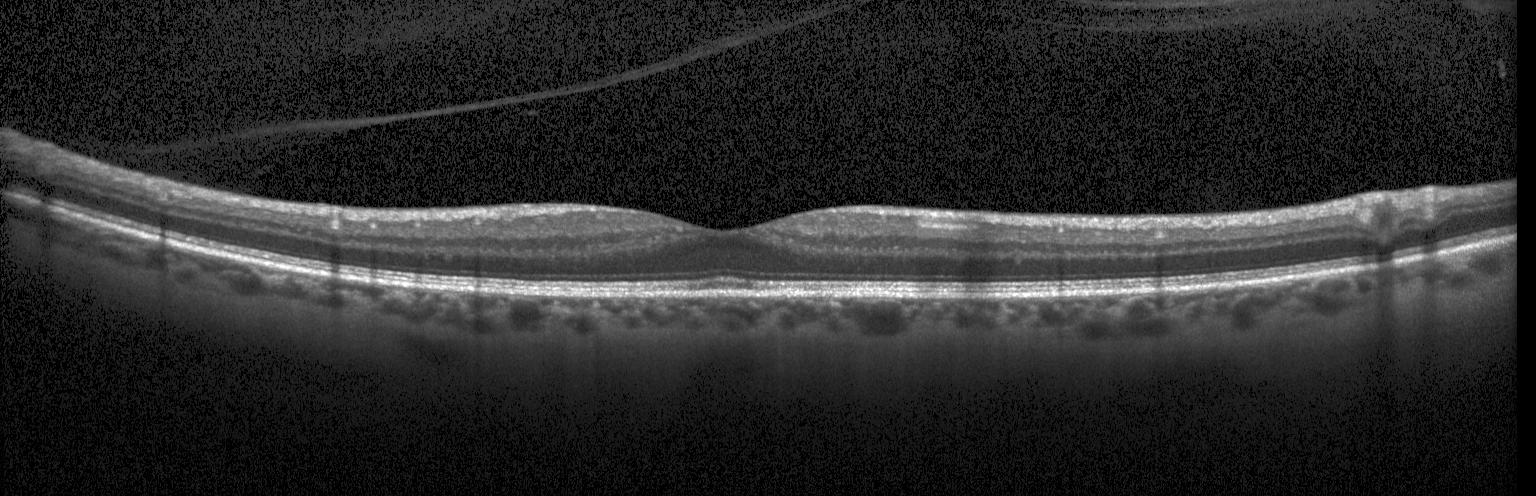
Optical coherence tomography scan; spectral-domain OCT; macular scan; Heidelberg Spectralis OCT system — Impression: no CNV, no DME, and no drusen.